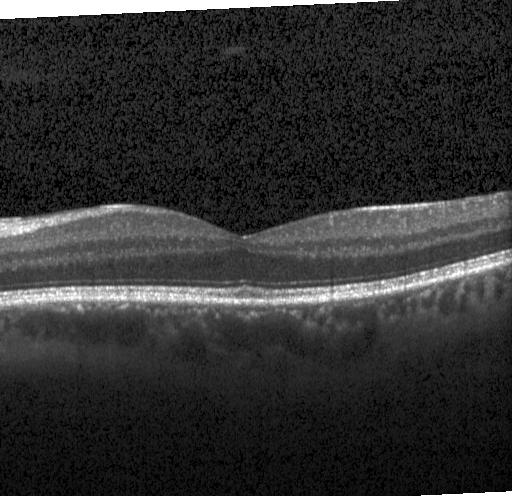
SD-OCT. OCT line scan. Heidelberg Spectralis OCT system
Impression: no choroidal neovascularization, diabetic macular edema, or drusen.